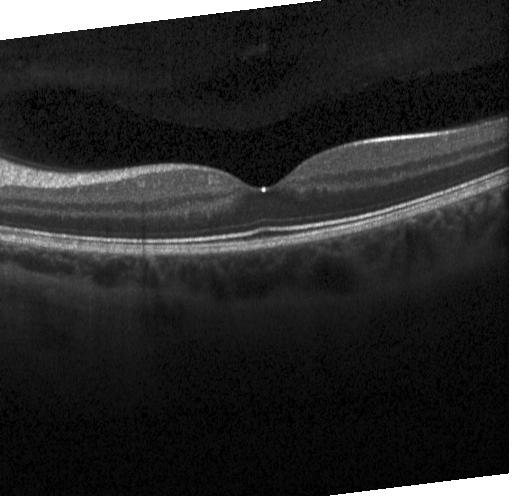

Retinal OCT cross-section · Heidelberg Spectralis — Finding: no CNV, no DME, and no drusen.